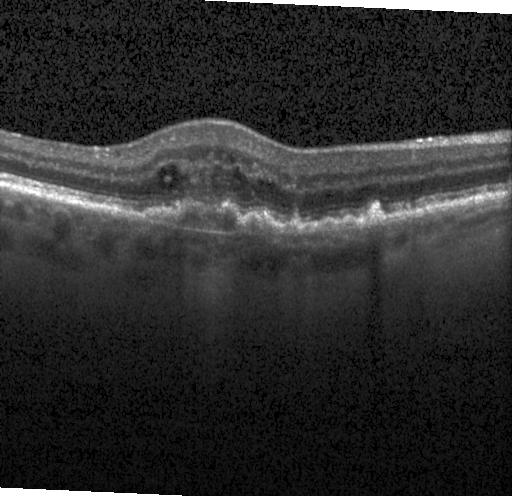 Spectral-domain OCT, retinal OCT cross-section.
A choroidal neovascular membrane.